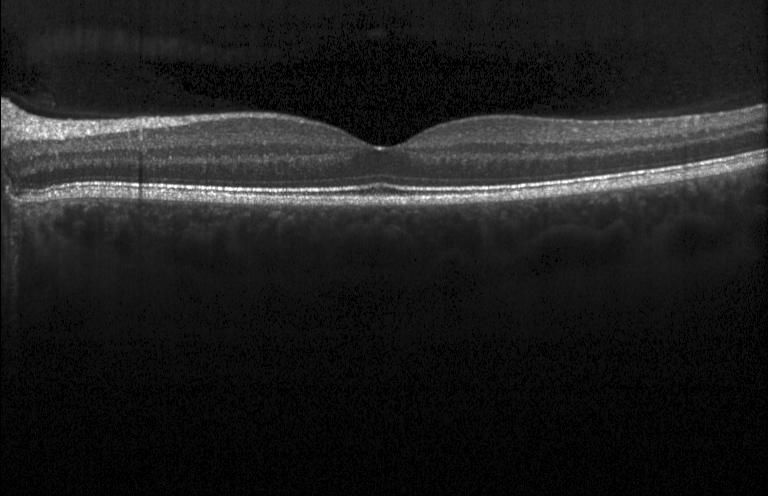 SD-OCT, OCT line scan, macular scan, acquired on a Heidelberg Spectralis. Diagnosis: neither choroidal neovascularization, diabetic macular edema, nor drusen.